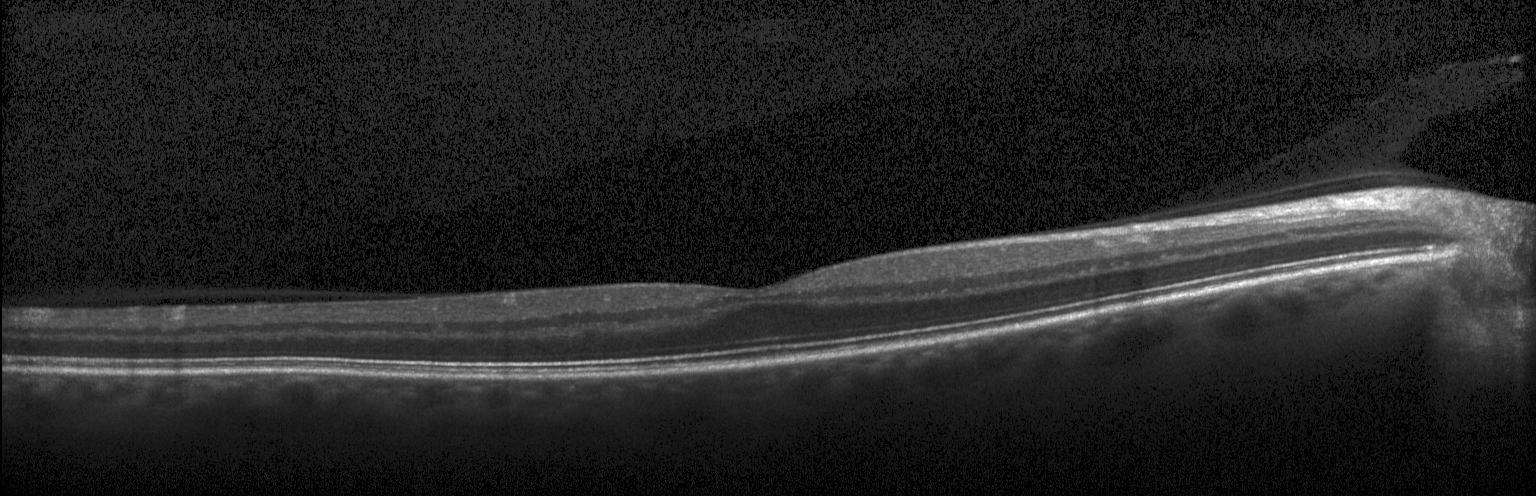

This B-scan demonstrates no CNV, DME, or drusen.